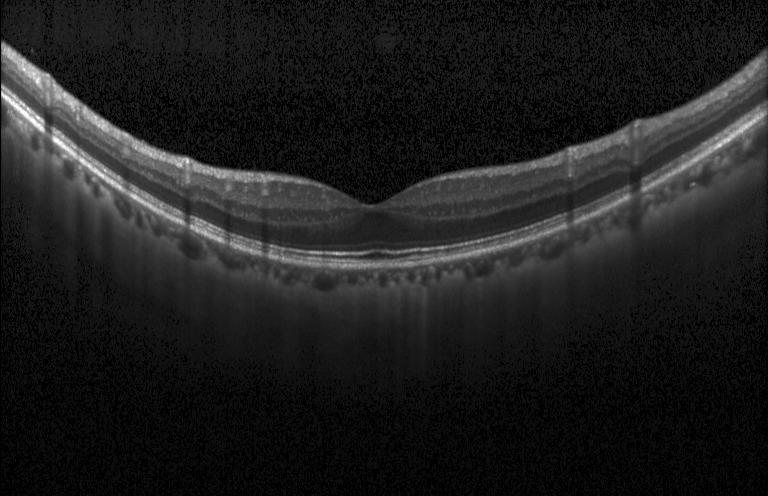
Impression: no CNV, DME, or drusen.